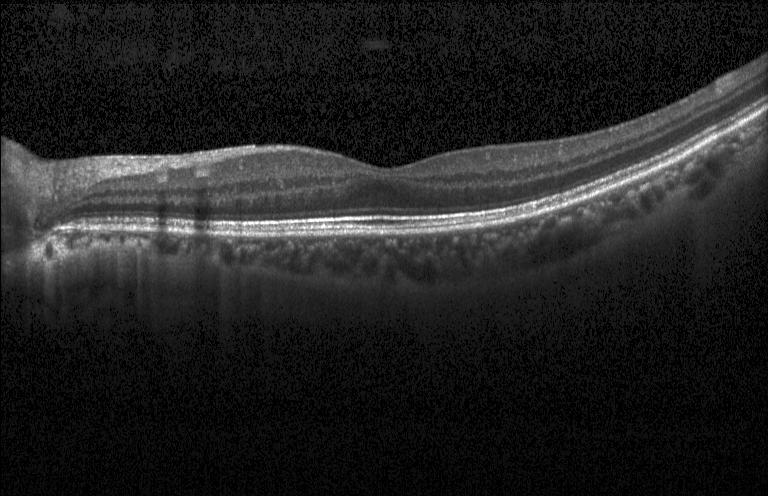

OCT B-scan · Heidelberg Spectralis OCT system · macular scan · spectral-domain OCT
OCT finding: no choroidal neovascularization, no diabetic macular edema, and no drusen.